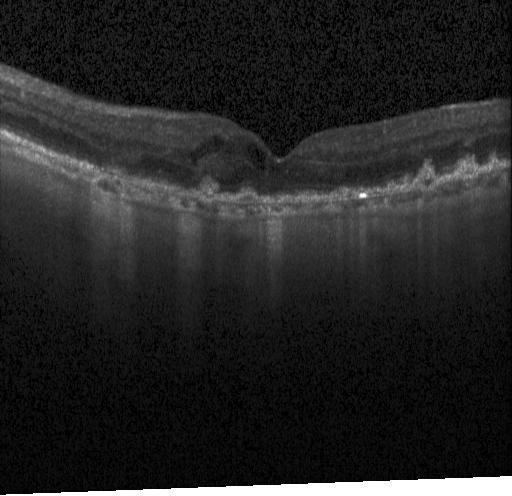

Retinal OCT cross-section · SD-OCT.
Finding: a choroidal neovascular membrane.